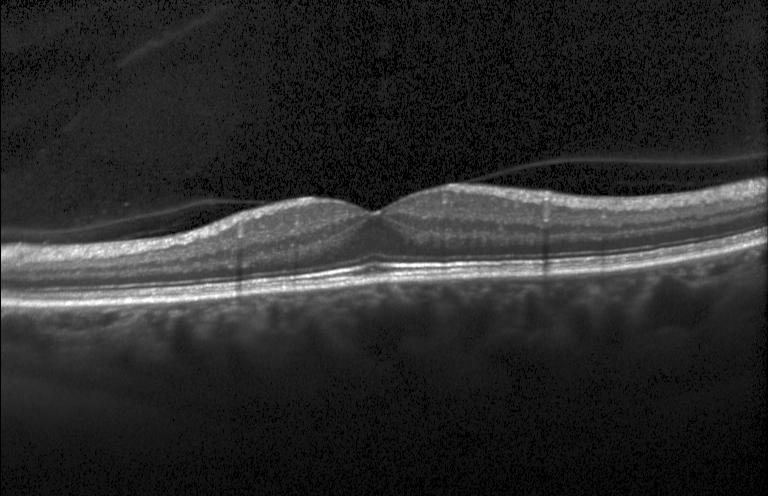

SD-OCT, Heidelberg Spectralis OCT system, retinal OCT cross-section, through the macula.
This B-scan demonstrates no choroidal neovascularization, no diabetic macular edema, and no drusen.